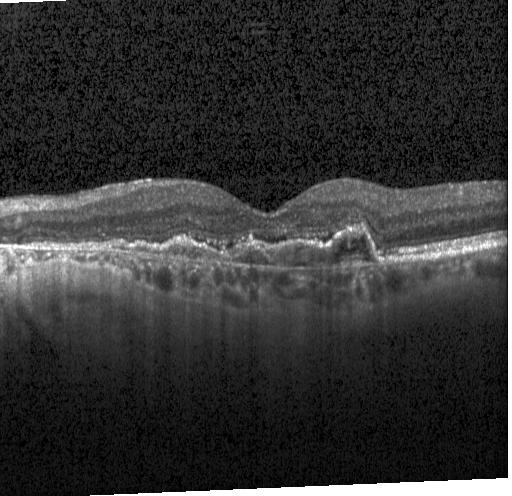
OCT B-scan; instrument: Heidelberg Spectralis; SD-OCT — Finding: choroidal neovascularization.